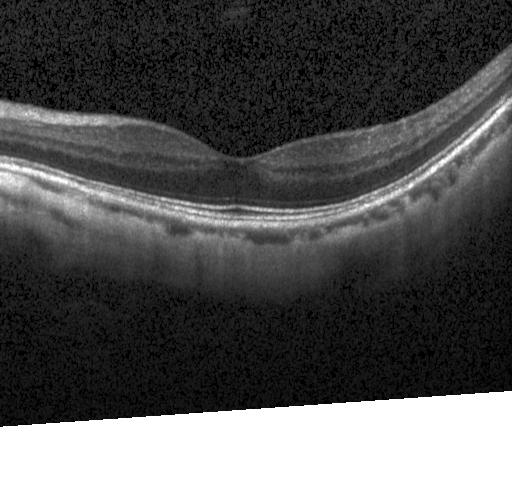

SD-OCT · horizontal scan through the fovea · OCT B-scan · Heidelberg Spectralis — The scan shows no choroidal neovascularization, diabetic macular edema, or drusen.